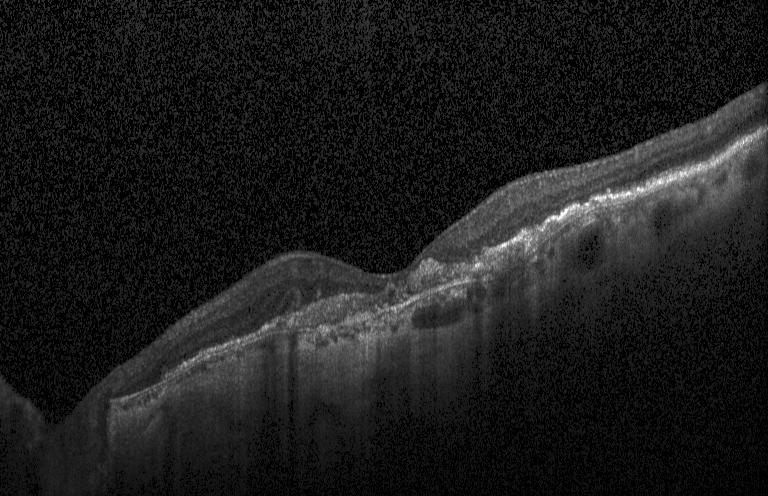 Horizontal scan through the fovea, OCT line scan, SD-OCT — Assessment: CNV.